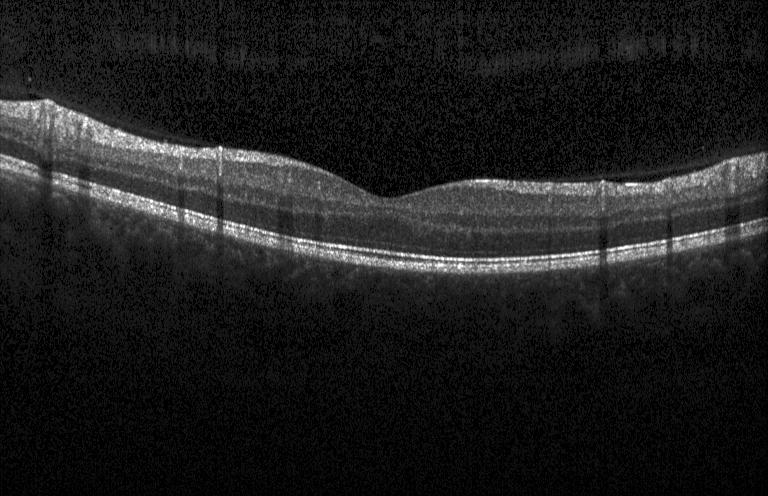
OCT B-scan showing neither choroidal neovascularization, diabetic macular edema, nor drusen.